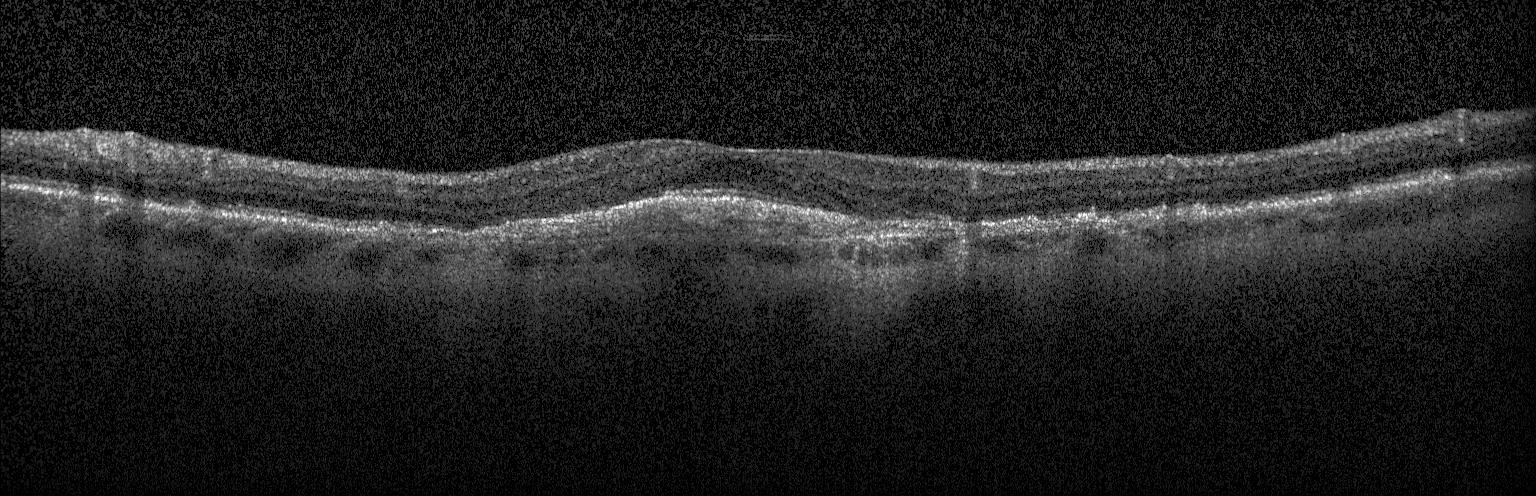 Optical coherence tomography B-scan; horizontal scan through the fovea
CNV.